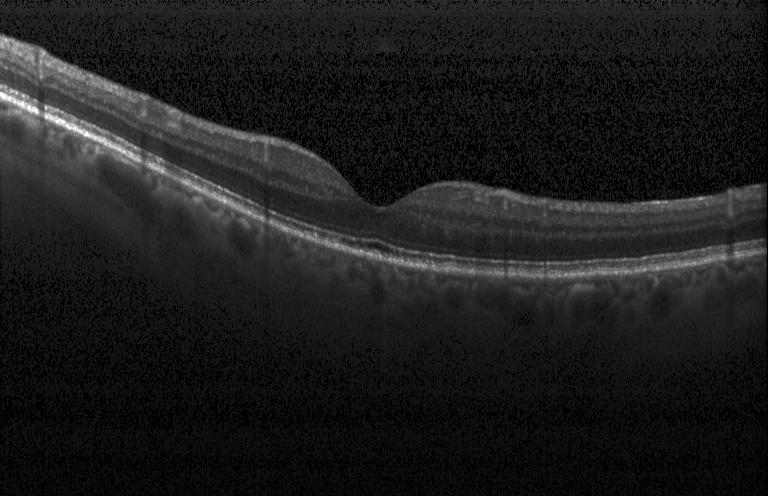 SD-OCT, optical coherence tomography scan.
The scan shows no evidence of choroidal neovascularization, diabetic macular edema, or drusen.